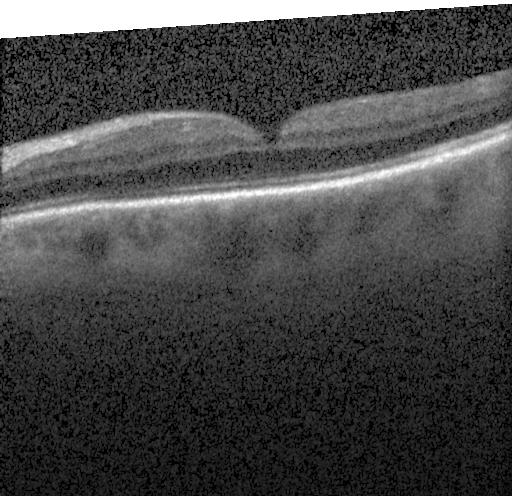 OCT finding: no evidence of choroidal neovascularization, diabetic macular edema, or drusen.